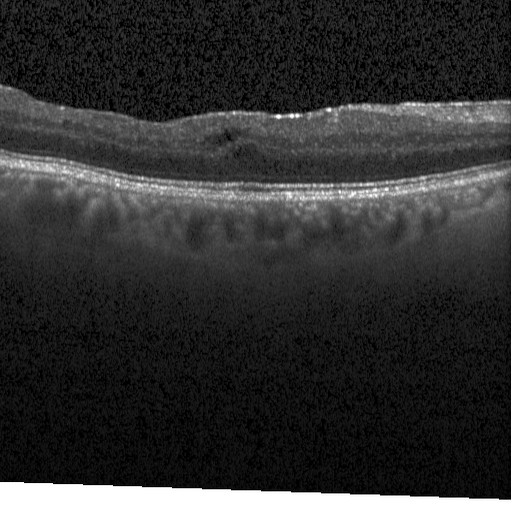
Macular OCT demonstrating DME.